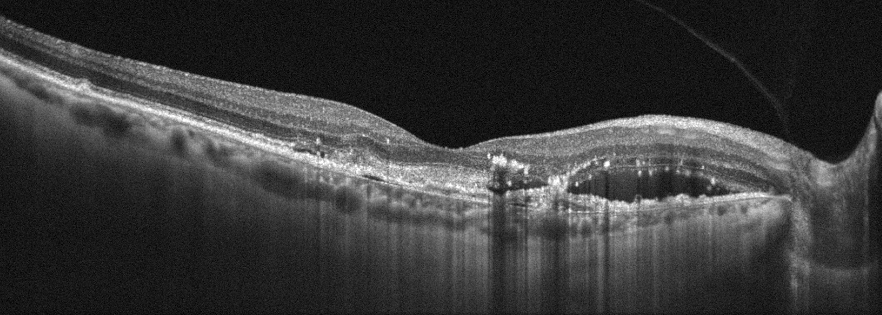

This B-scan demonstrates age-related macular degeneration (AMD).